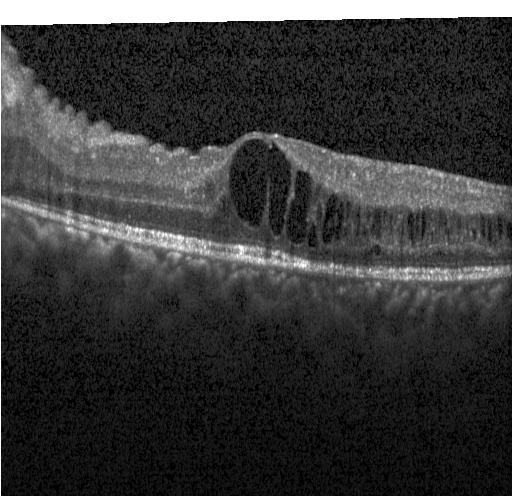

Optical coherence tomography scan. Acquired on a Heidelberg Spectralis. This B-scan demonstrates diabetic macular edema (DME).